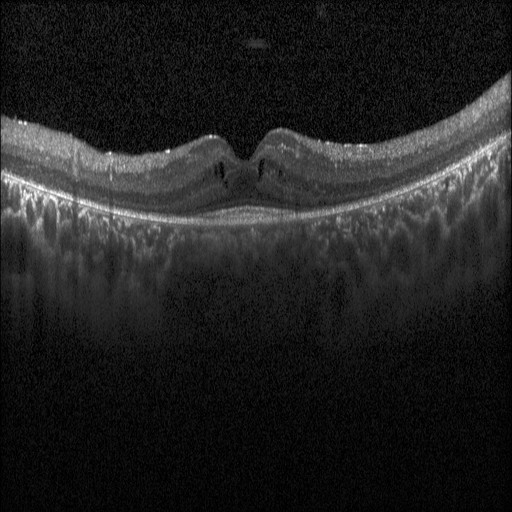 The scan shows diabetic macular edema.